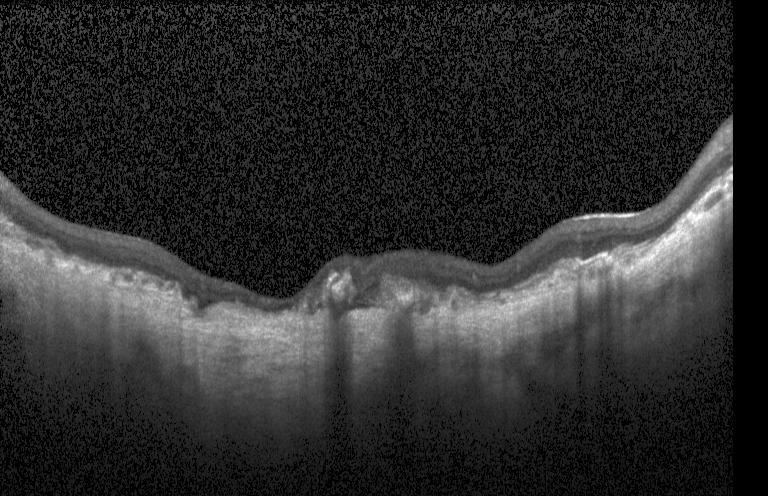

Dx: a choroidal neovascular membrane.